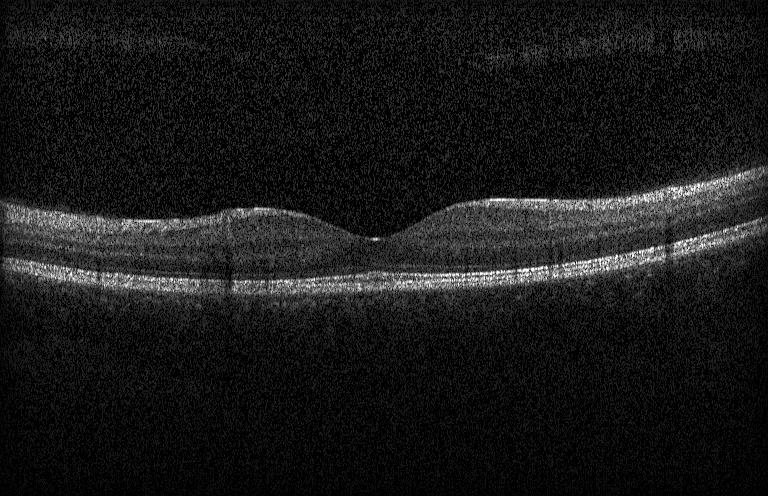 Diagnosis: neither CNV, DME, nor drusen.